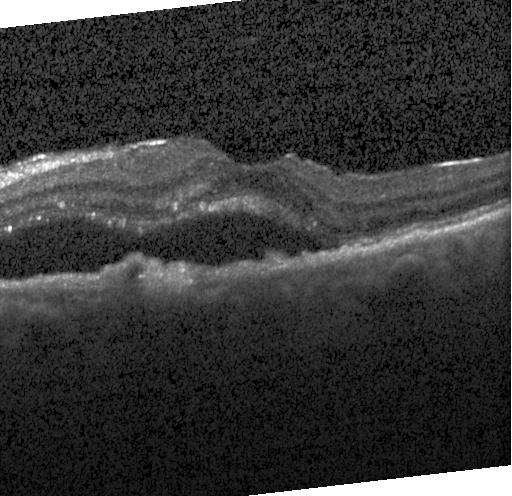

Retinal OCT cross-section showing a choroidal neovascular membrane.